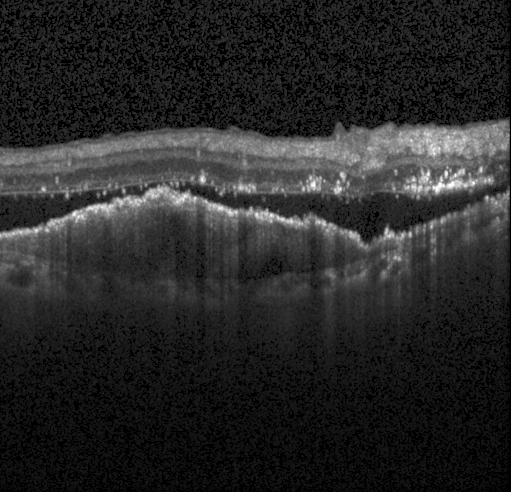 Optical coherence tomography scan.
Assessment: a choroidal neovascular membrane.